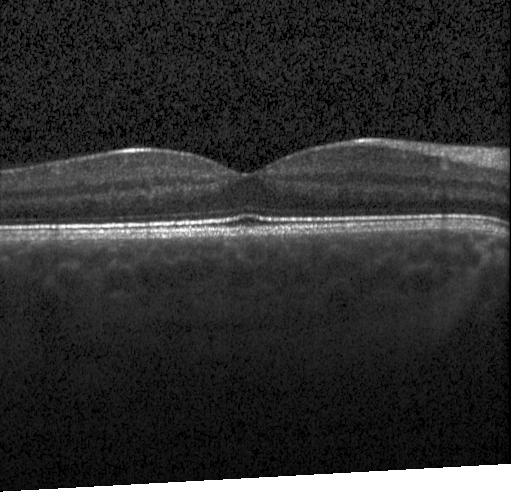 Spectral-domain OCT, OCT line scan, horizontal scan through the fovea — No choroidal neovascularization, diabetic macular edema, or drusen.